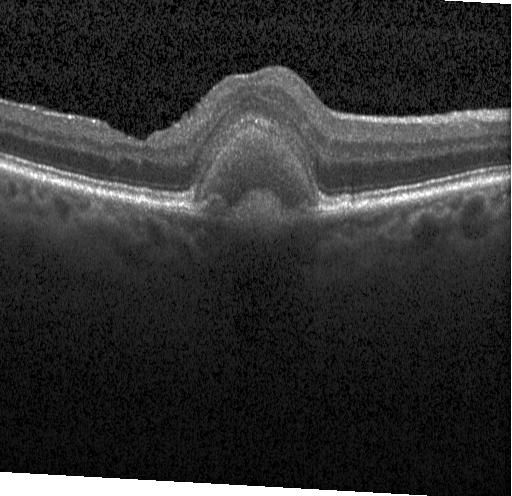

Retinal OCT cross-section.
Assessment: CNV.